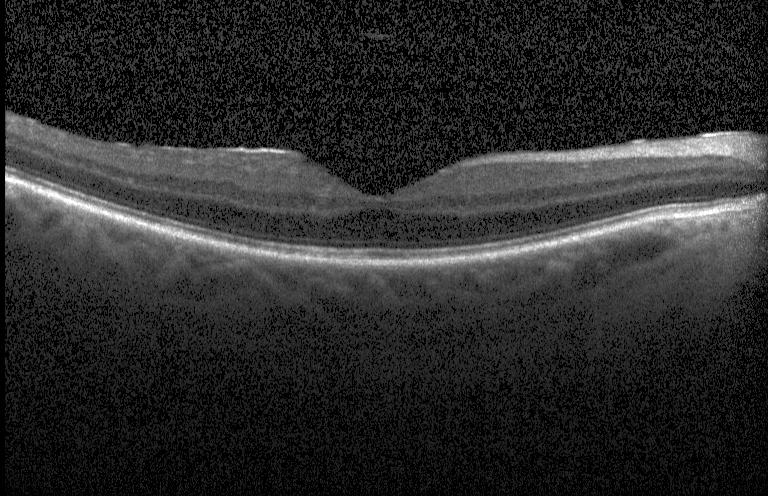 OCT B-scan. Heidelberg Spectralis OCT system
Diagnosis: no choroidal neovascularization, no diabetic macular edema, and no drusen.